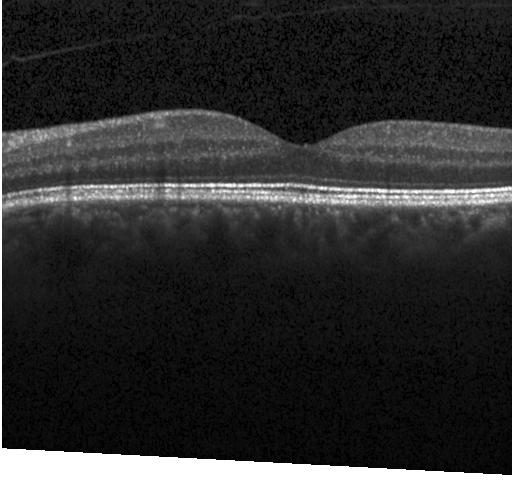
Assessment: no choroidal neovascularization, diabetic macular edema, or drusen.